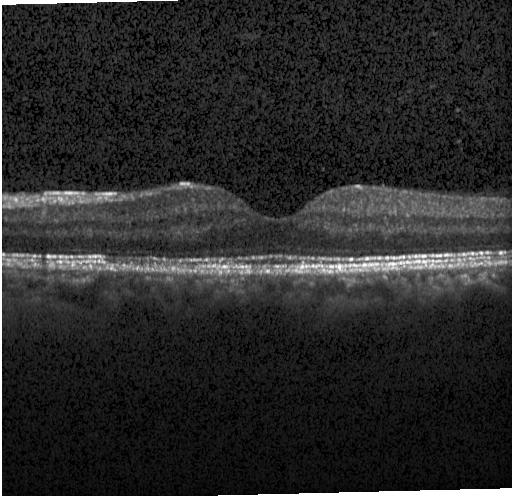 Assessment: no CNV, no DME, and no drusen.